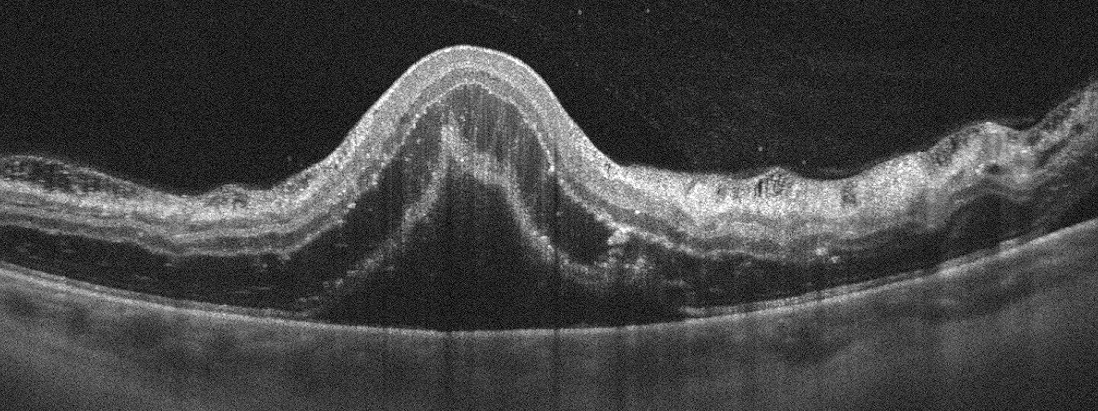 OCT line scan. Diagnosis: retinal vein occlusion.